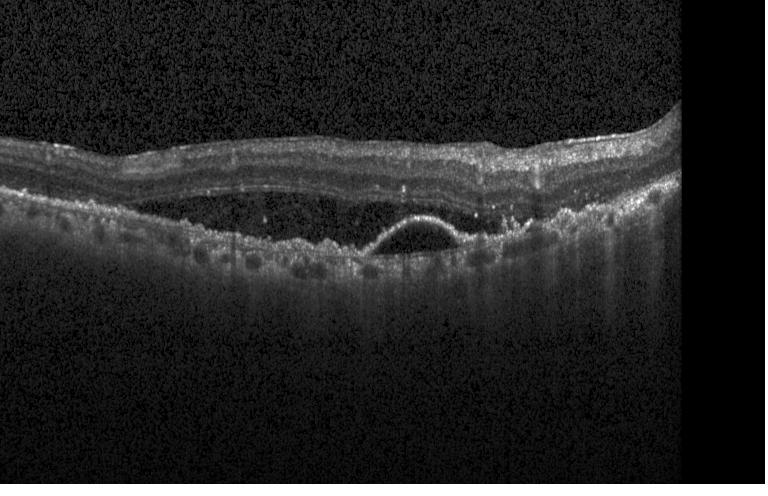
Retinal OCT cross-section, macular scan, spectral-domain optical coherence tomography, acquired on a Heidelberg Spectralis — Macular OCT: a choroidal neovascular membrane.